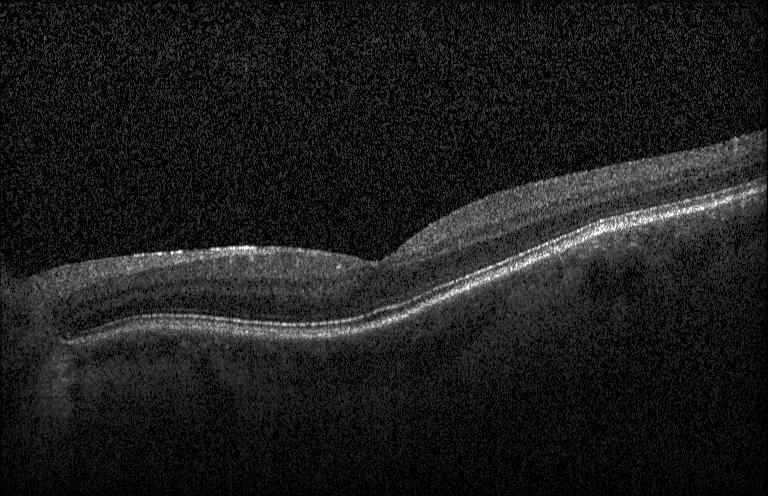

Retinal OCT cross-section.
Diagnosis: no evidence of choroidal neovascularization, diabetic macular edema, or drusen.